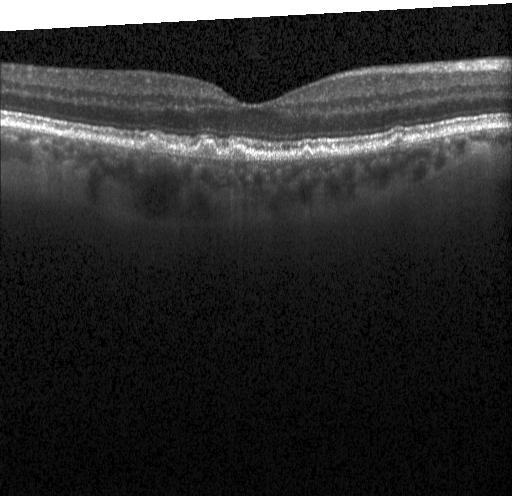

Macular OCT demonstrating sub-RPE drusenoid deposits.